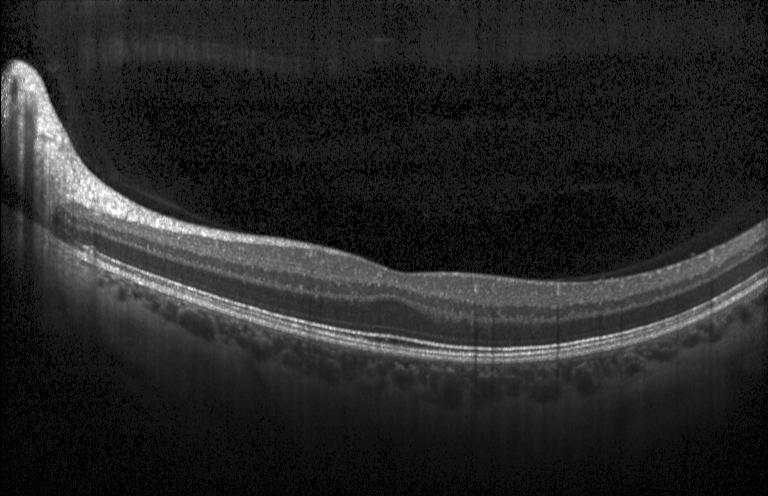 Heidelberg Spectralis; horizontal scan through the fovea; optical coherence tomography B-scan
Diagnosis: no choroidal neovascularization, no diabetic macular edema, and no drusen.